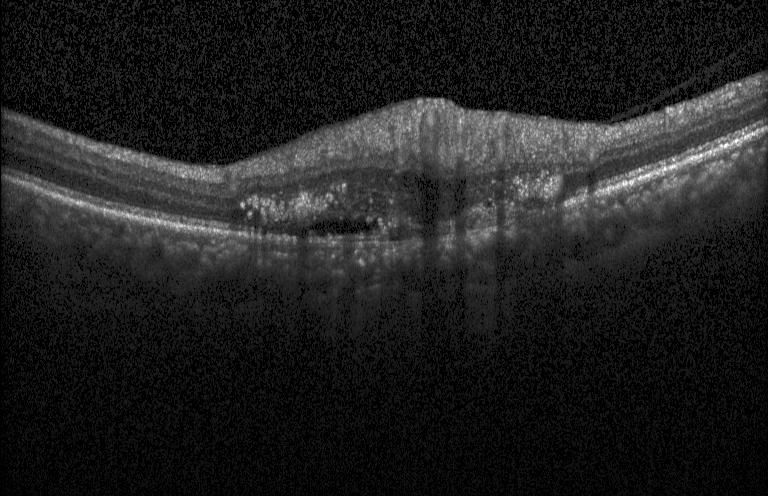 Horizontal scan through the fovea, spectral-domain OCT, Heidelberg Spectralis, retinal OCT B-scan.
Macular OCT: choroidal neovascularization (CNV).